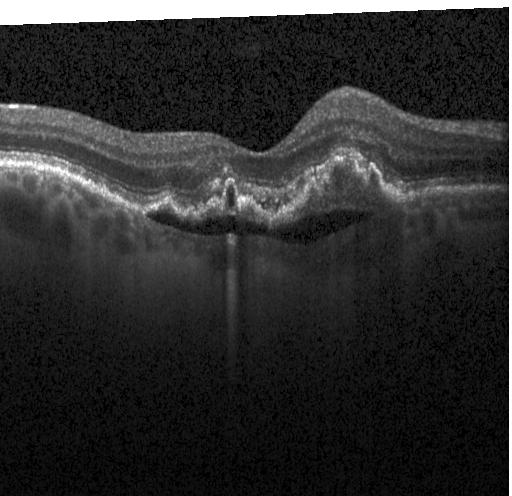

Macular OCT demonstrating choroidal neovascularization.